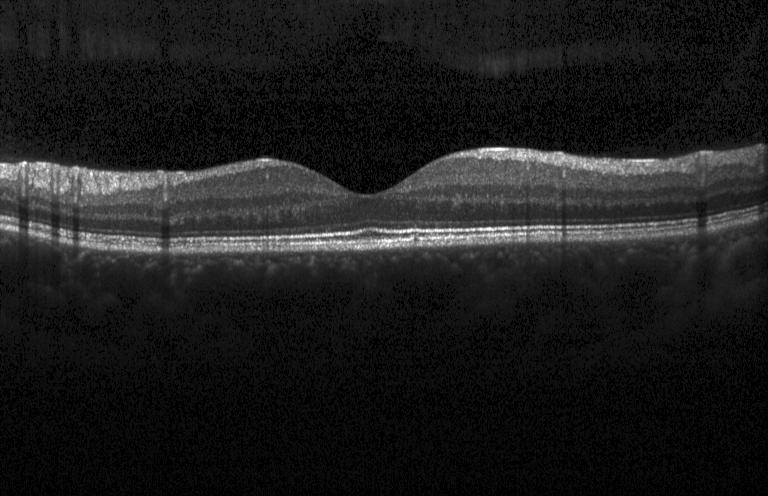 Spectral-domain OCT; optical coherence tomography scan. Macular OCT: no CNV, DME, or drusen.